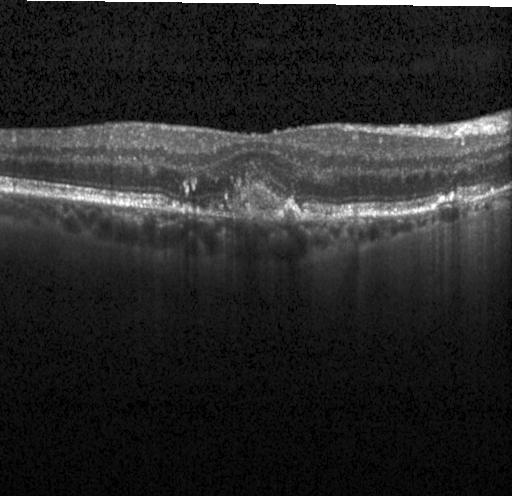 This B-scan demonstrates choroidal neovascularization.